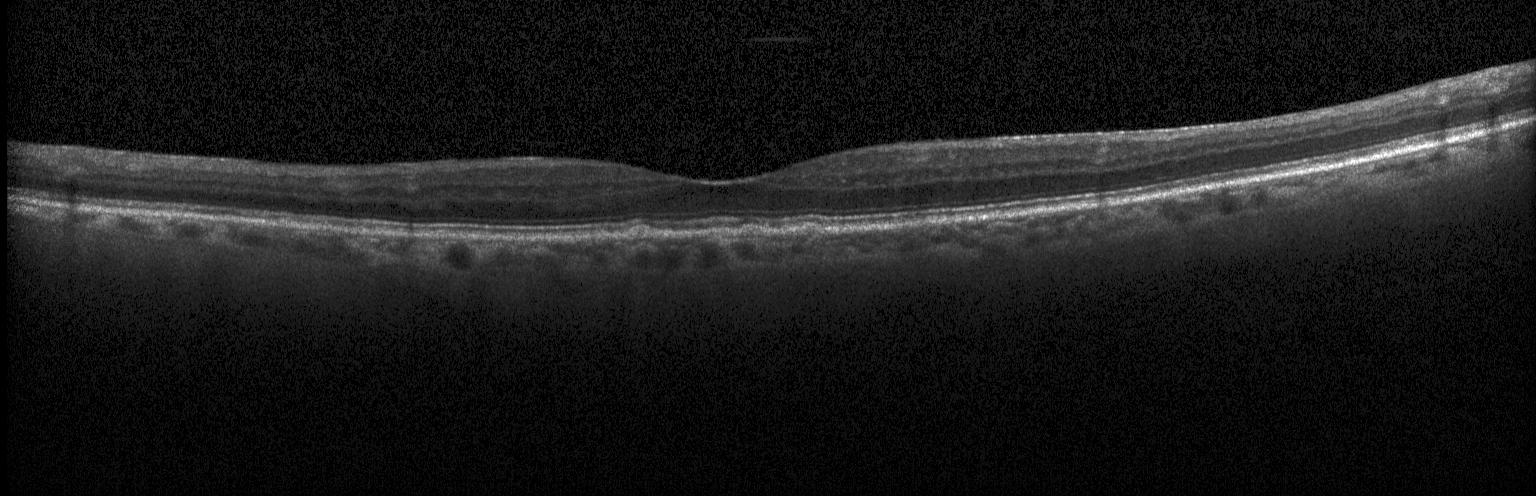

Retinal OCT B-scan
This B-scan demonstrates sub-RPE drusenoid deposits.